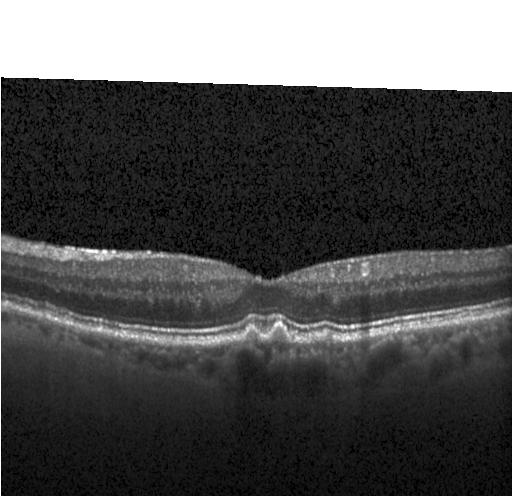 Spectral-domain optical coherence tomography; retinal OCT cross-section; horizontal scan through the fovea — Impression: drusen.